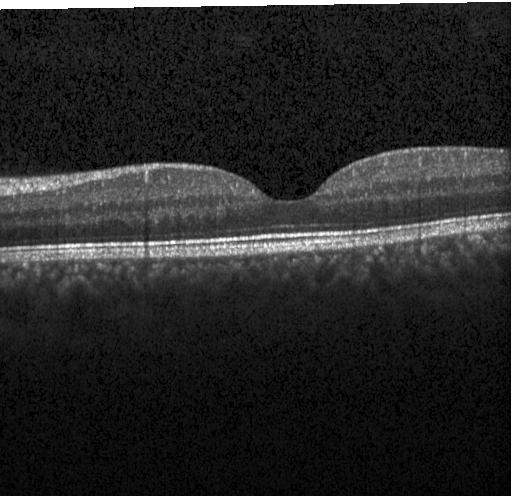
Horizontal scan through the fovea · retinal OCT B-scan · SD-OCT — Diagnosis: neither choroidal neovascularization, diabetic macular edema, nor drusen.